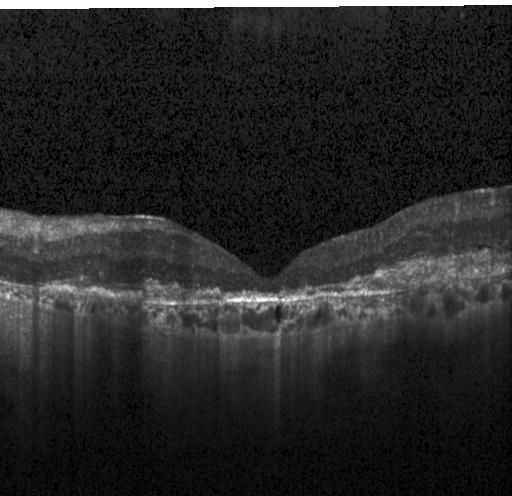

SD-OCT; fovea-centered; OCT line scan — Diagnosis: a choroidal neovascular membrane.